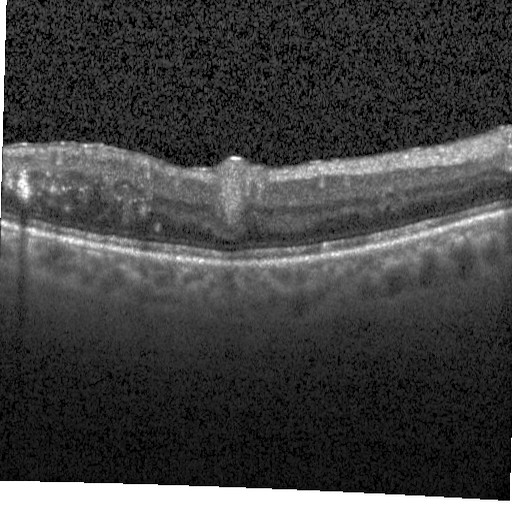

OCT line scan. Heidelberg Spectralis OCT system. Spectral-domain OCT.
This B-scan demonstrates DME.